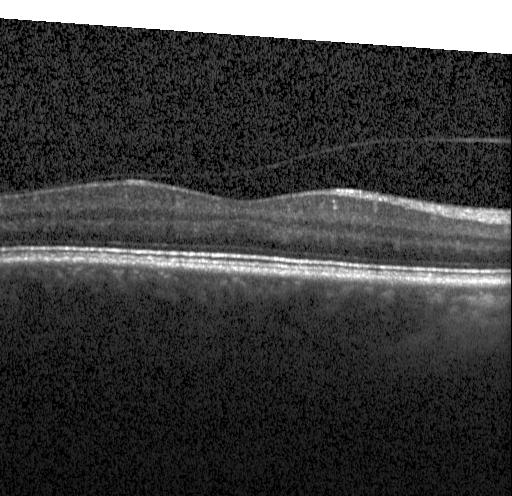 SD-OCT; retinal OCT cross-section; macular scan; Heidelberg Spectralis. Finding: no CNV, DME, or drusen.